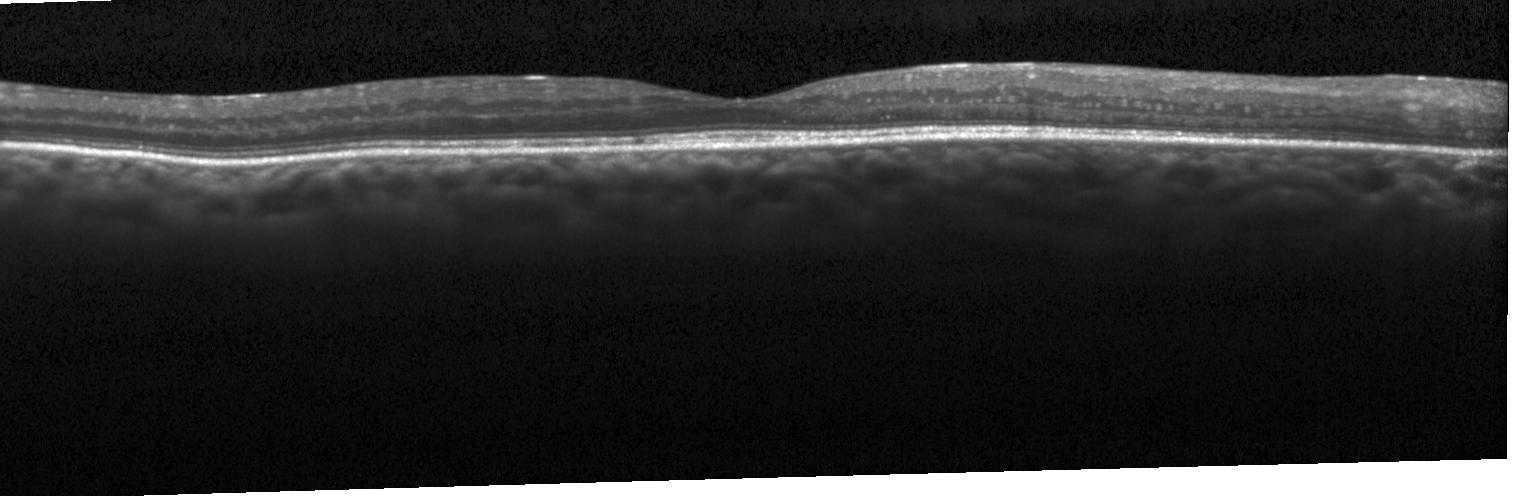

Optical coherence tomography B-scan; Heidelberg Spectralis OCT system; spectral-domain optical coherence tomography — The scan shows no choroidal neovascularization, diabetic macular edema, or drusen.